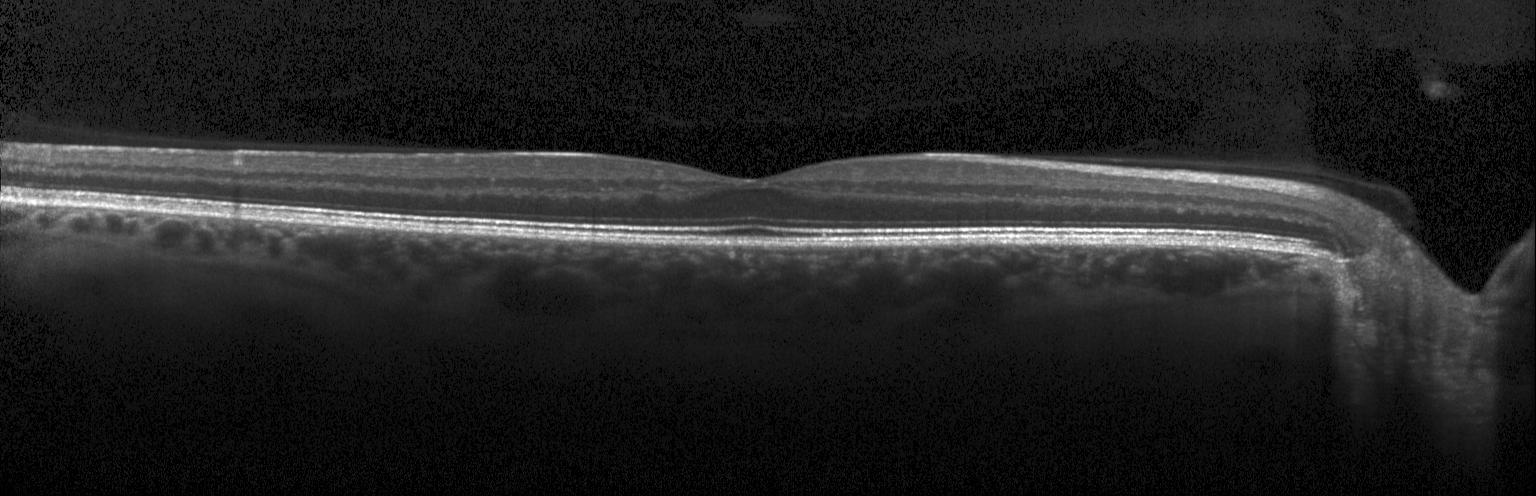 Heidelberg Spectralis OCT system, OCT B-scan — The scan shows neither choroidal neovascularization, diabetic macular edema, nor drusen.